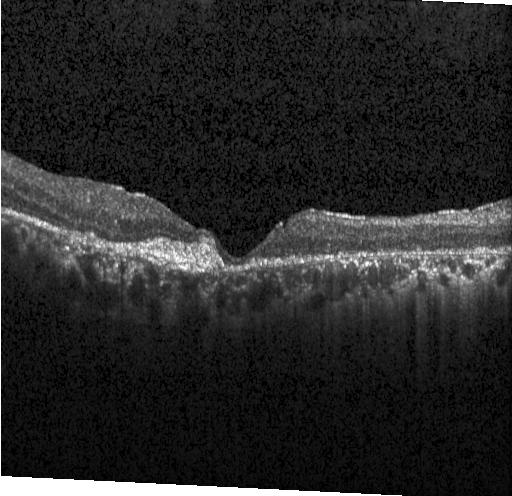

Instrument: Heidelberg Spectralis. Retinal OCT cross-section. Fovea-centered. Spectral-domain OCT
The scan shows choroidal neovascularization.